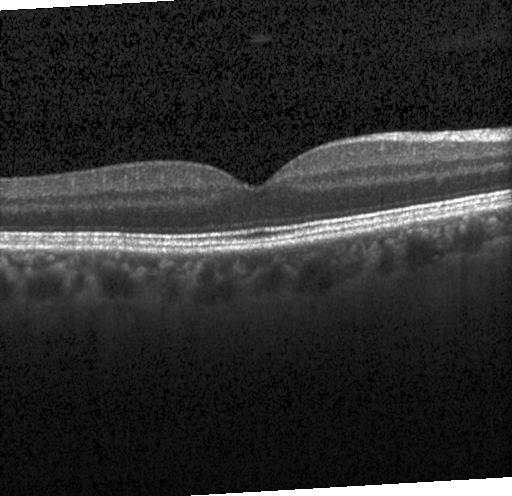 Retinal OCT cross-section, centered on the fovea, SD-OCT. Macular OCT: neither CNV, DME, nor drusen.